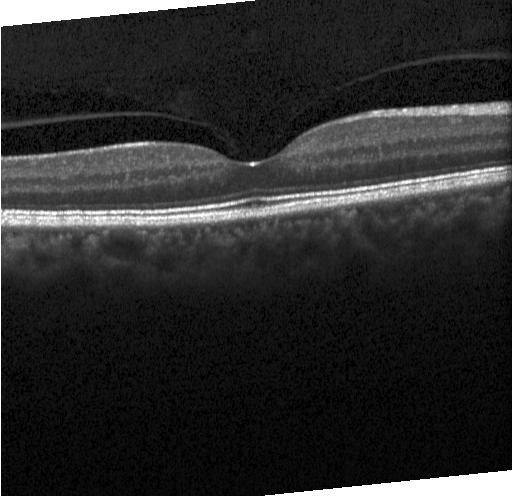 Retinal OCT B-scan
Diagnosis: no evidence of CNV, DME, or drusen.